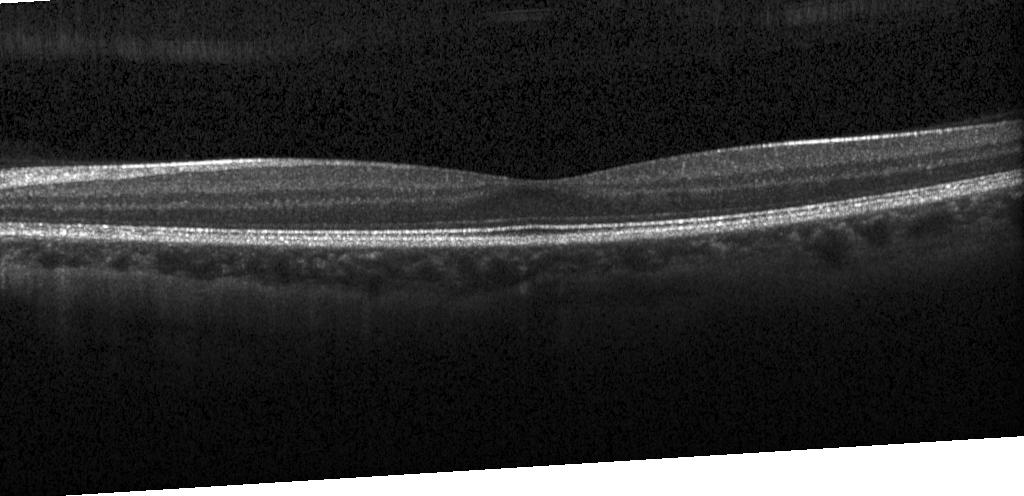

Finding: no CNV, DME, or drusen.